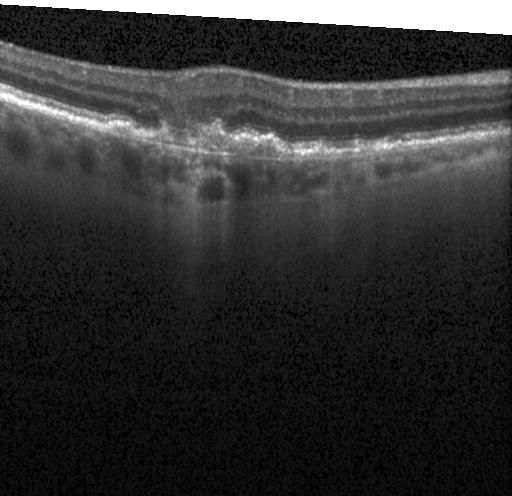

Retinal OCT cross-section showing a choroidal neovascular membrane.